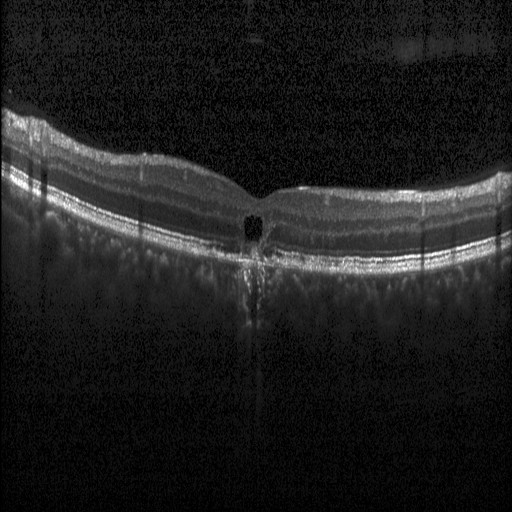
Spectral-domain OCT; optical coherence tomography B-scan; macular scan — OCT finding: diabetic macular edema.